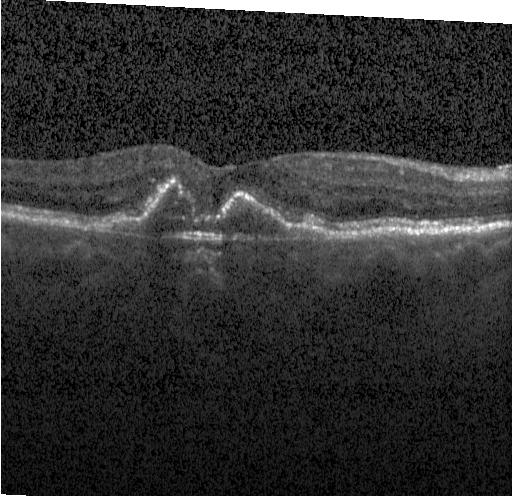
Optical coherence tomography scan · fovea-centered · Heidelberg Spectralis OCT system.
A choroidal neovascular membrane.